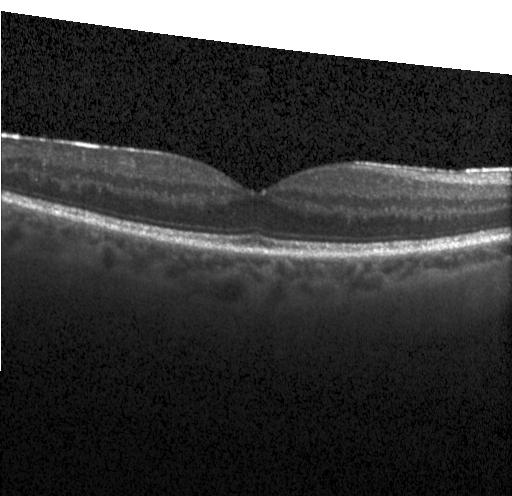
Impression: neither CNV, DME, nor drusen.